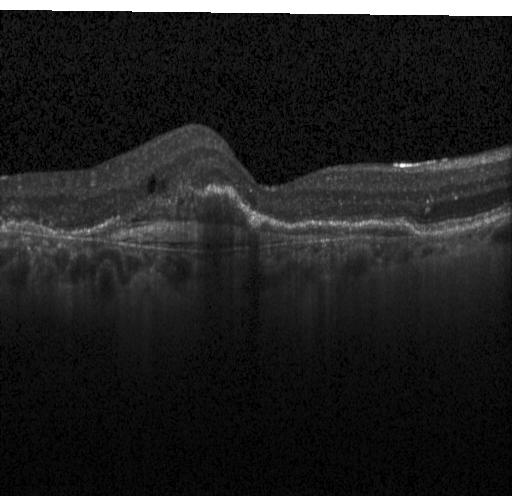 Retinal OCT cross-section
Dx: choroidal neovascularization (CNV).